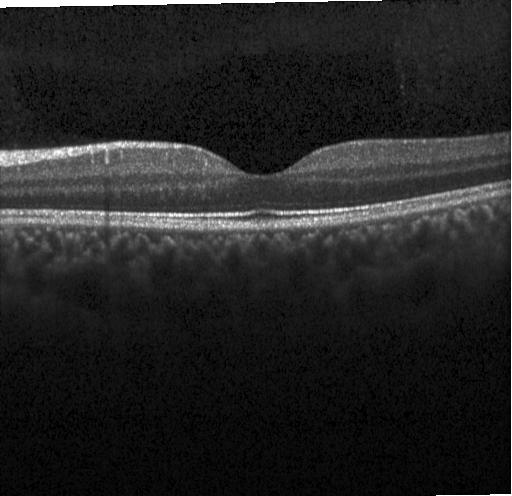 No evidence of choroidal neovascularization, diabetic macular edema, or drusen.